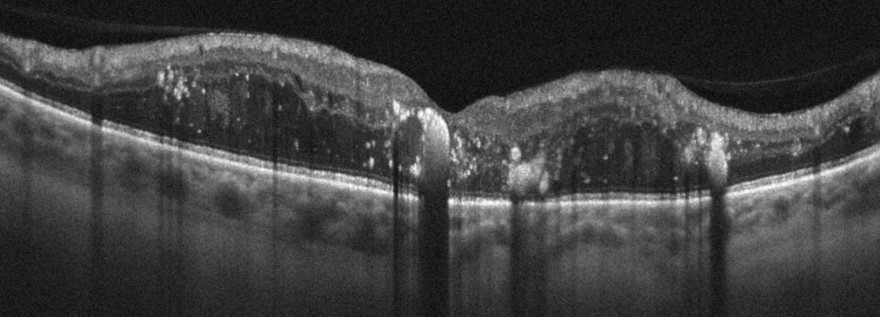 Optical coherence tomography scan.
Dx: diabetic macular edema (DME).